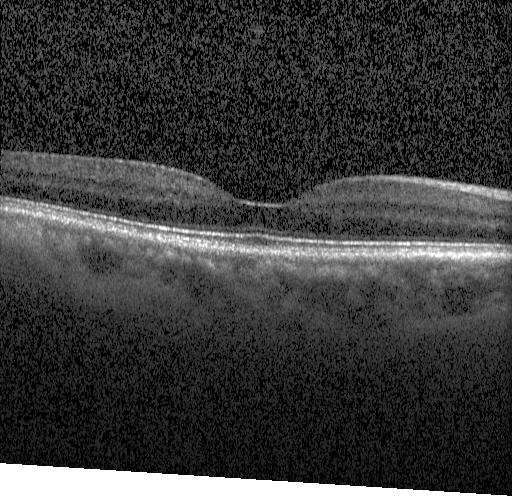
OCT finding: no evidence of choroidal neovascularization, diabetic macular edema, or drusen.